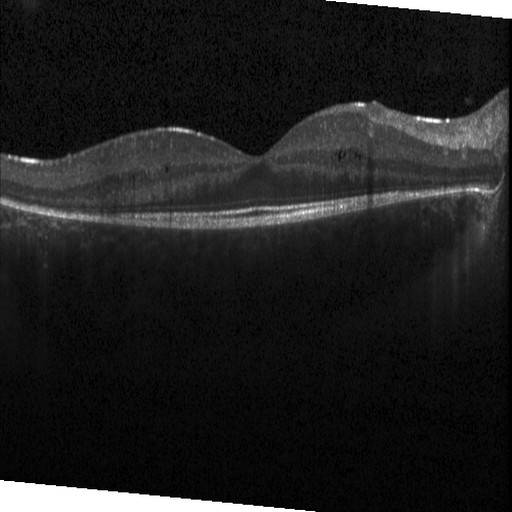
SD-OCT · Heidelberg Spectralis · macular scan · retinal OCT B-scan. Assessment: DME.